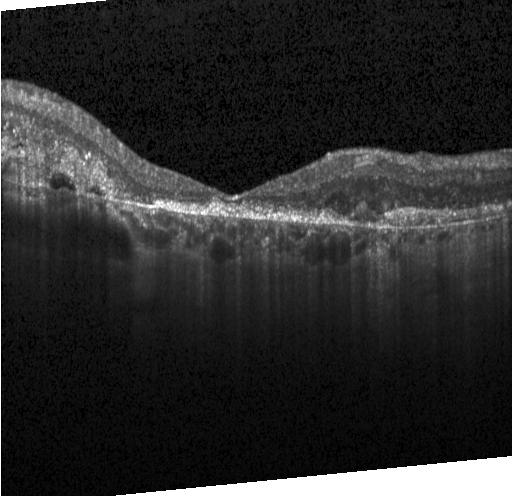 OCT line scan.
Impression: a choroidal neovascular membrane.